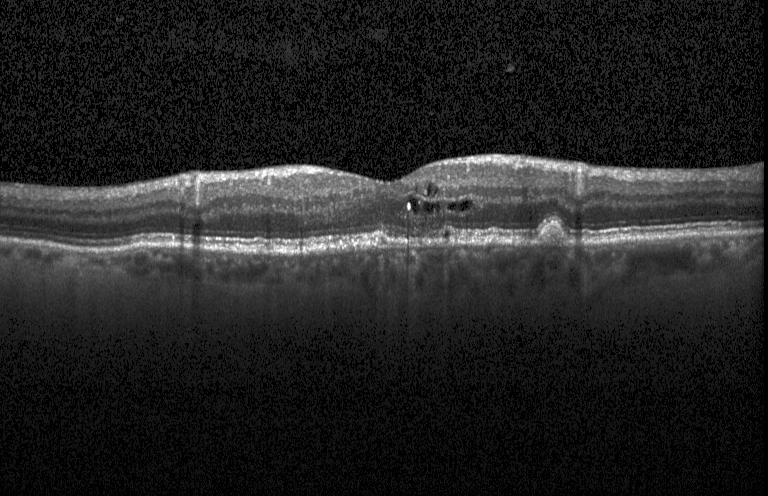 Retinal OCT cross-section. Acquired on a Heidelberg Spectralis
Finding: a choroidal neovascular membrane.